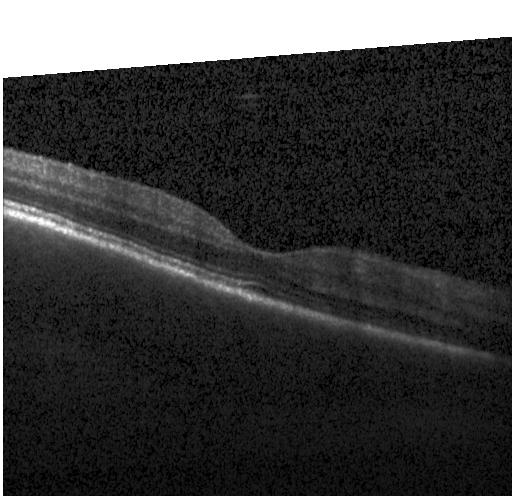 Dx: no evidence of choroidal neovascularization, diabetic macular edema, or drusen.